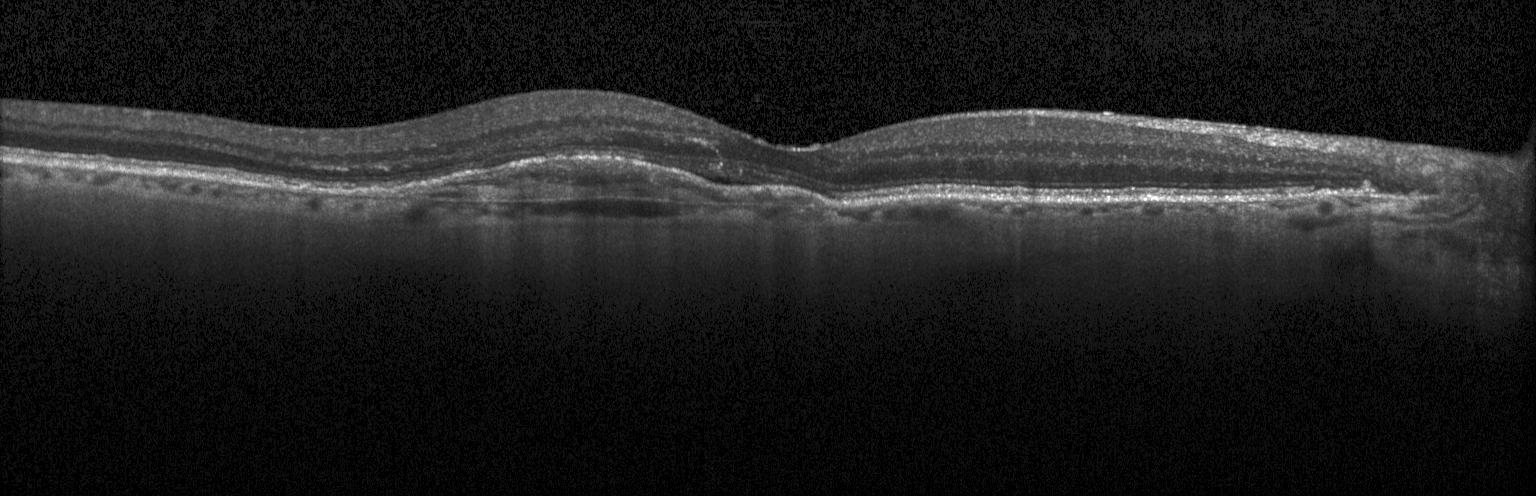 OCT line scan. Spectral-domain OCT. Instrument: Heidelberg Spectralis. Through the macula — Diagnosis: a choroidal neovascular membrane.